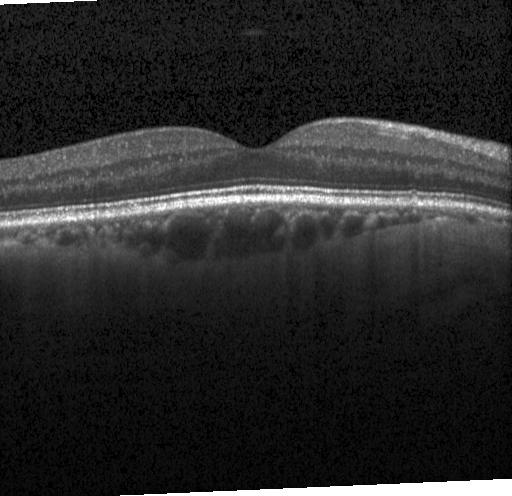

SD-OCT · OCT line scan · through the macula — Assessment: drusen.